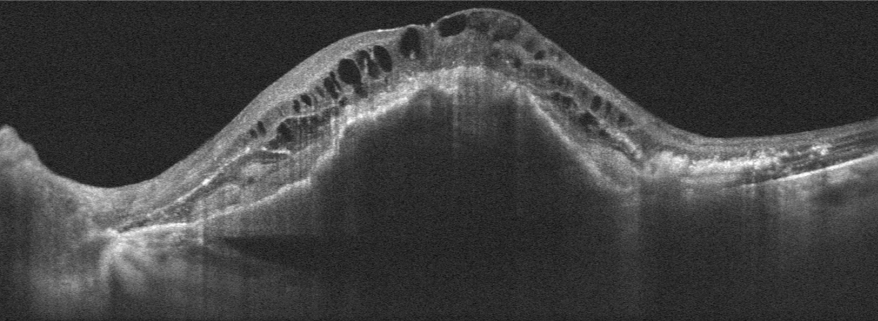
Impression: age-related macular degeneration.